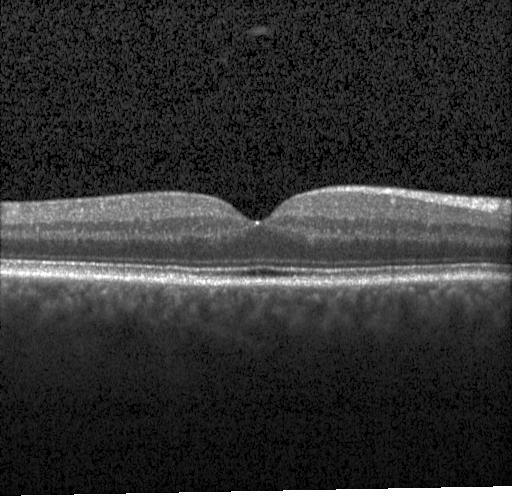

Heidelberg Spectralis · through the macula · optical coherence tomography scan. Neither choroidal neovascularization, diabetic macular edema, nor drusen.